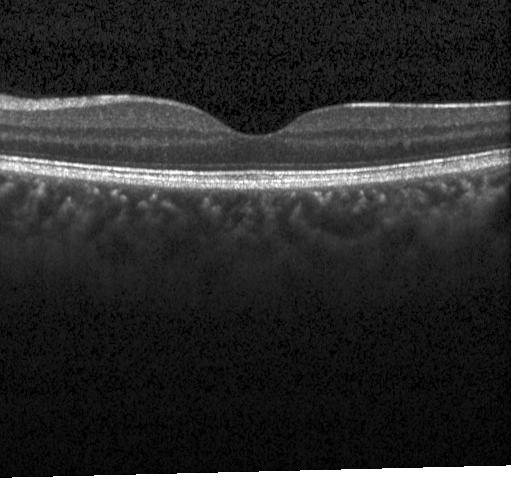

Optical coherence tomography scan.
Diagnosis: no CNV, no DME, and no drusen.